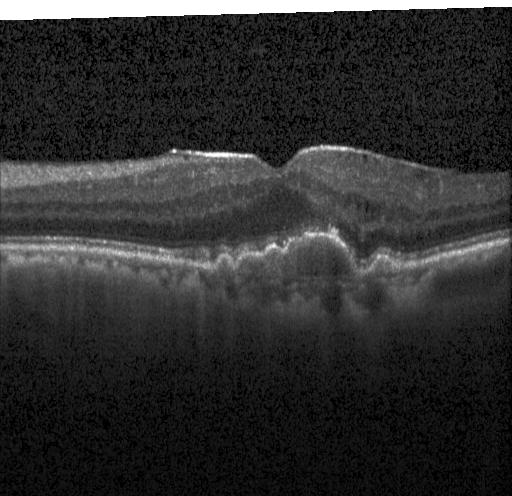 Through the macula. Optical coherence tomography scan. SD-OCT. Instrument: Heidelberg Spectralis — Assessment: choroidal neovascularization (CNV).